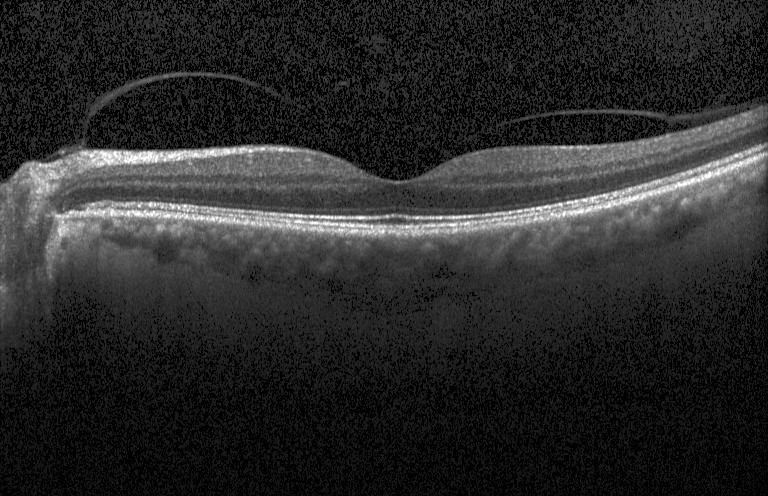

SD-OCT. Optical coherence tomography B-scan. Heidelberg Spectralis. Horizontal scan through the fovea — OCT finding: no choroidal neovascularization, diabetic macular edema, or drusen.